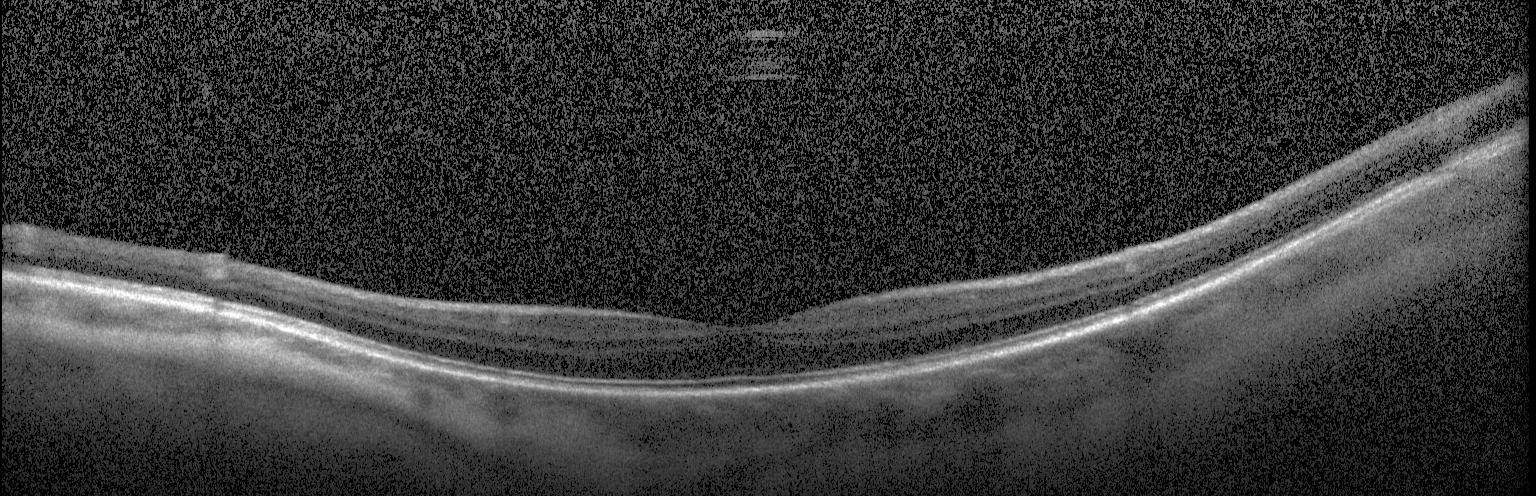 Macular OCT: no choroidal neovascularization, diabetic macular edema, or drusen.